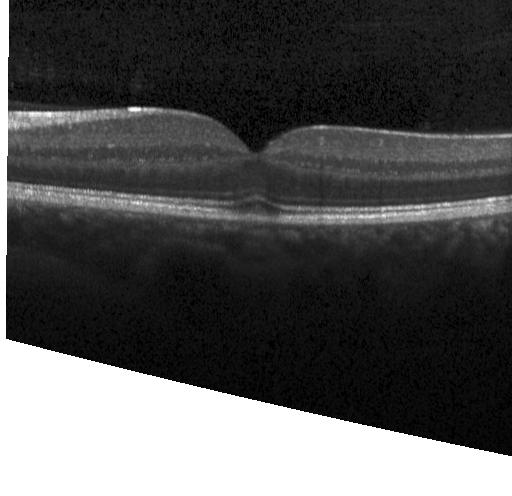 OCT line scan.
Assessment: no choroidal neovascularization, no diabetic macular edema, and no drusen.